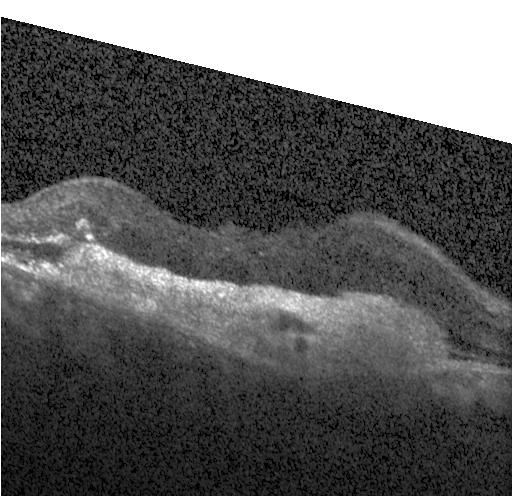 Heidelberg Spectralis OCT system. Macular scan. Optical coherence tomography B-scan. Spectral-domain optical coherence tomography — Finding: a choroidal neovascular membrane.